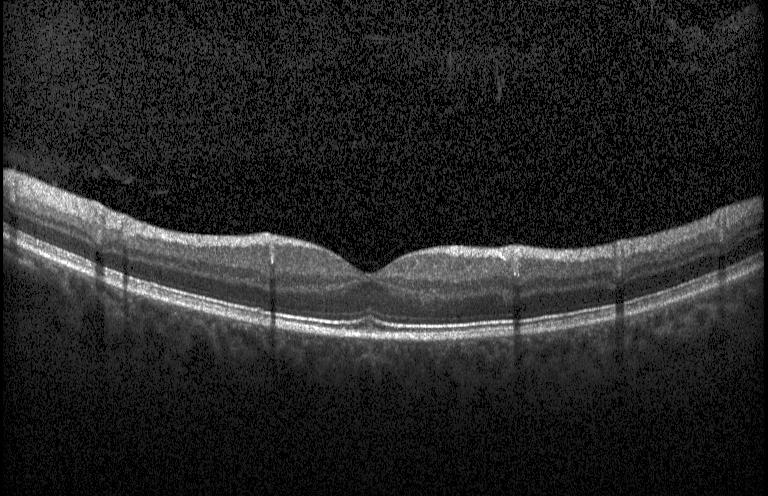

OCT line scan; spectral-domain OCT; acquired on a Heidelberg Spectralis; fovea-centered
No CNV, no DME, and no drusen.